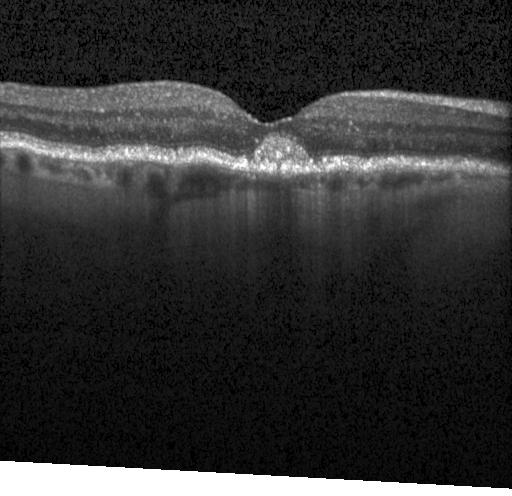

Assessment: multiple drusen.